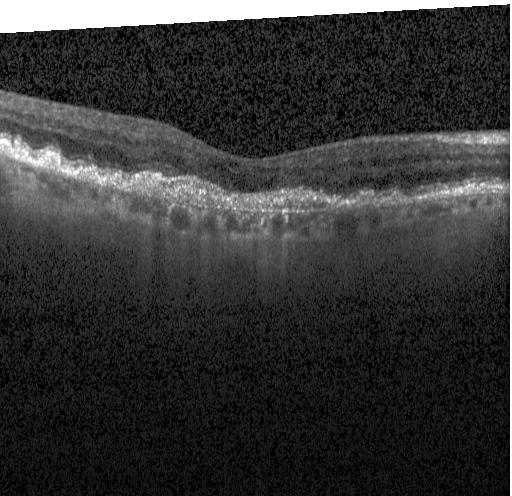

Dx: a choroidal neovascular membrane.